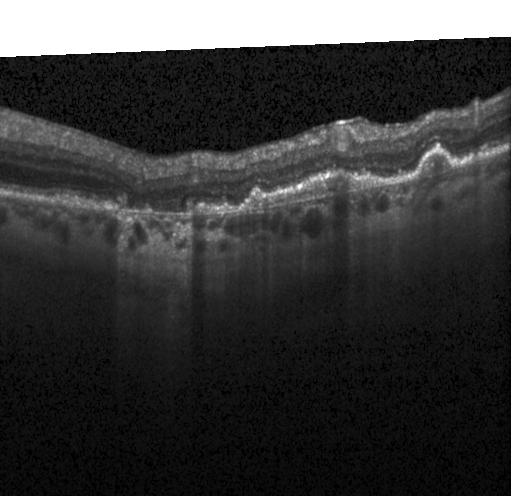 Assessment: choroidal neovascularization (CNV).